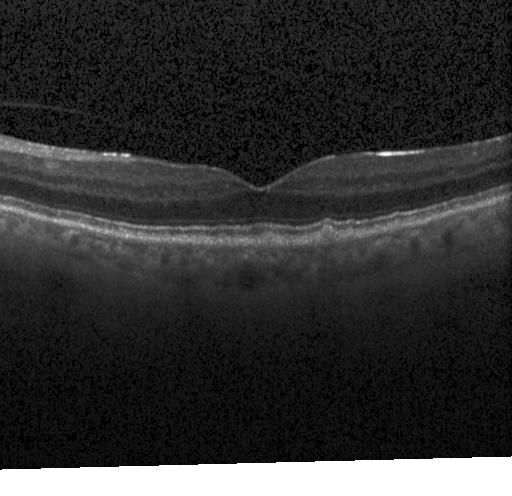 OCT finding: sub-RPE drusenoid deposits.